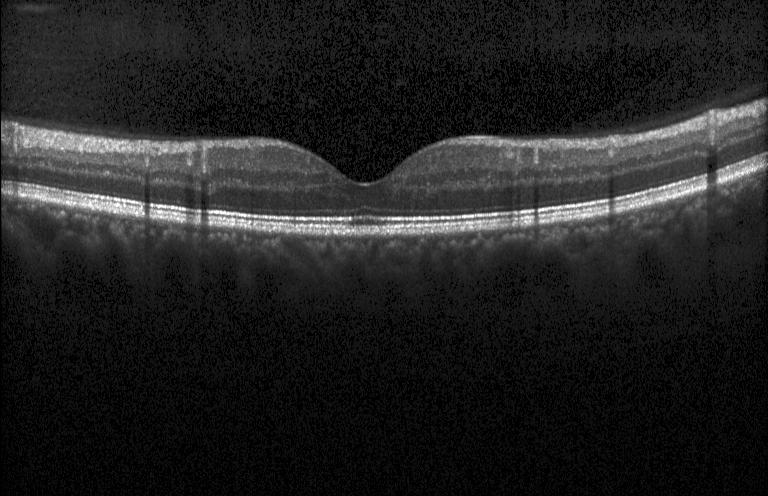
Optical coherence tomography scan, through the macula. This B-scan demonstrates no choroidal neovascularization, no diabetic macular edema, and no drusen.